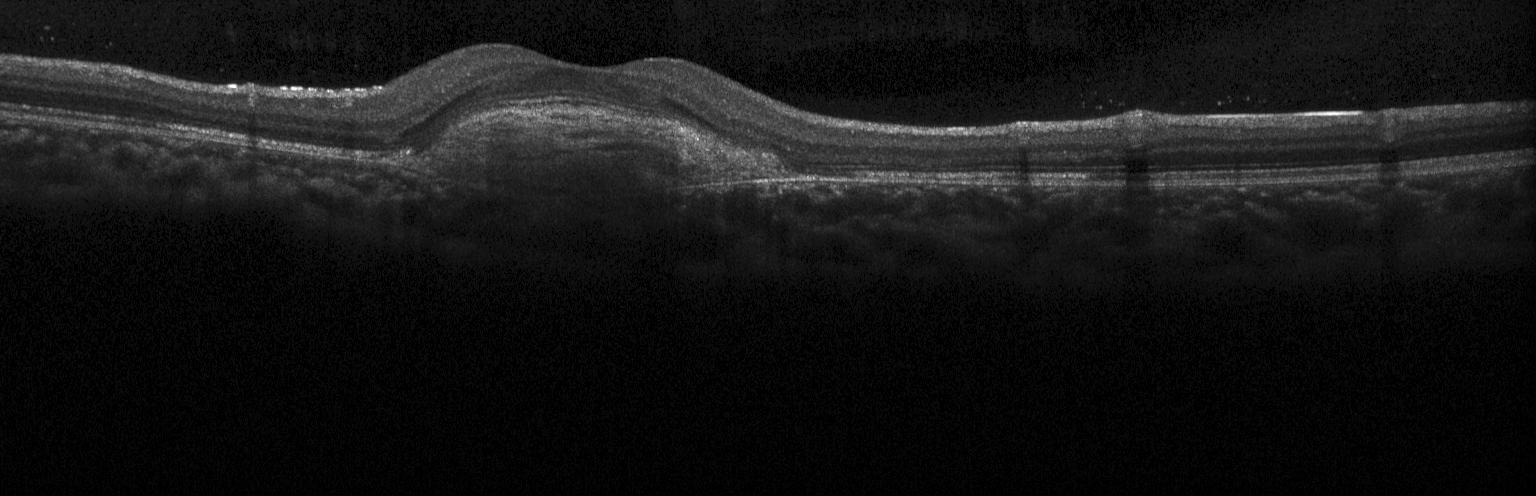 This B-scan demonstrates a choroidal neovascular membrane.